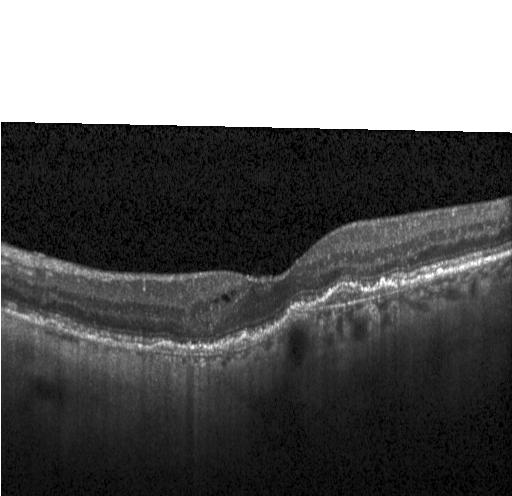

OCT B-scan. Acquired on a Heidelberg Spectralis — Assessment: a choroidal neovascular membrane.